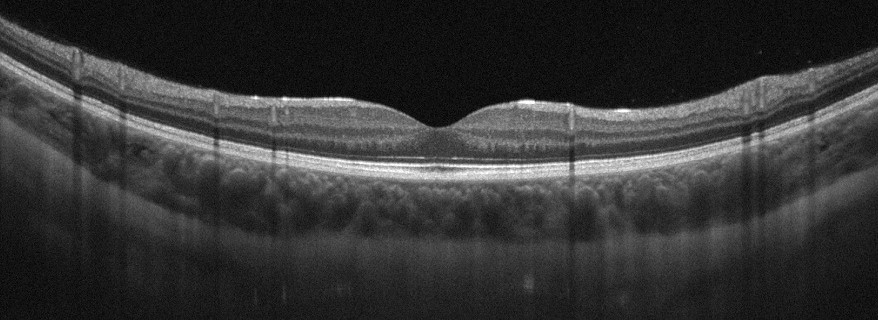 Retinal OCT cross-section showing no AMD, DME, ERM, RAO, RVO, or VID.